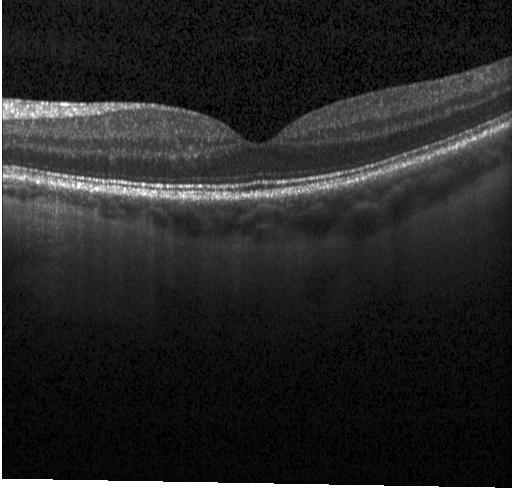

Spectral-domain optical coherence tomography · macular scan · optical coherence tomography B-scan
Impression: neither choroidal neovascularization, diabetic macular edema, nor drusen.